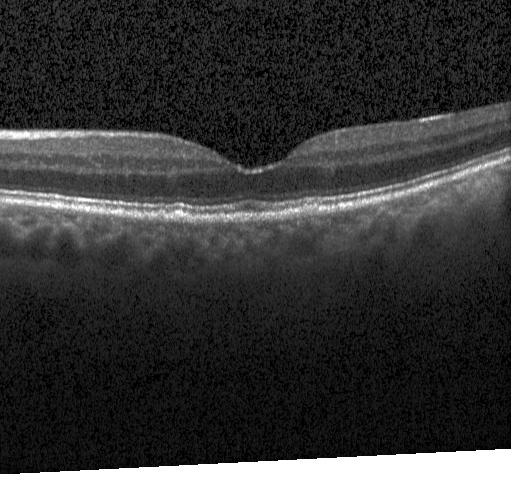 Spectral-domain OCT · retinal OCT B-scan · macular scan · instrument: Heidelberg Spectralis
Impression: drusen.